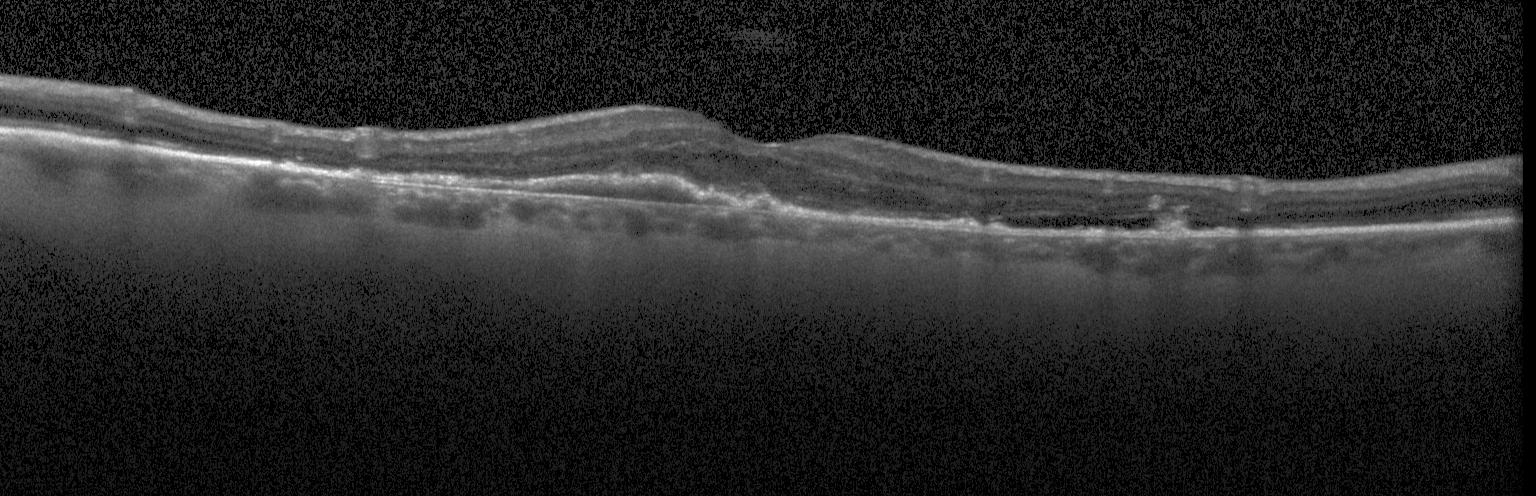 OCT finding: a choroidal neovascular membrane.